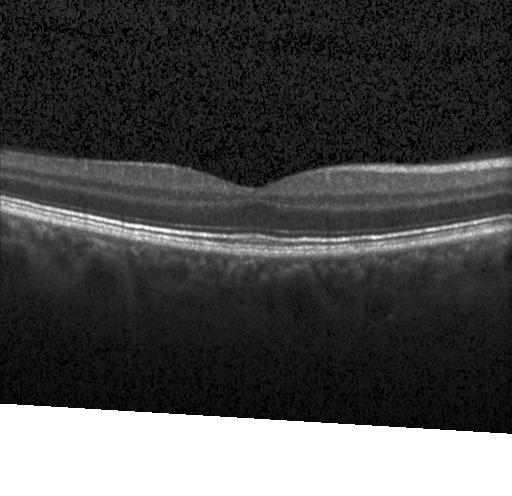

Dx: no choroidal neovascularization, diabetic macular edema, or drusen.